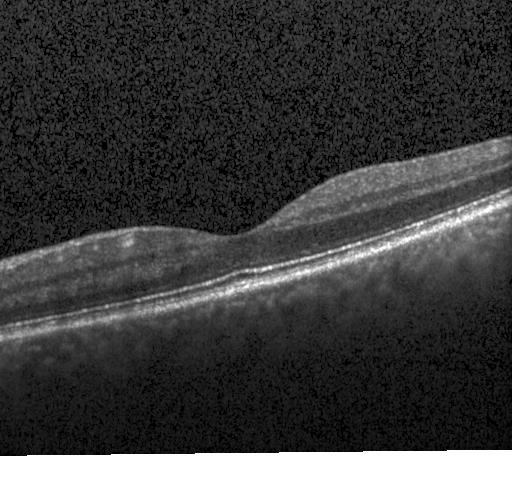 Impression: no evidence of choroidal neovascularization, diabetic macular edema, or drusen.